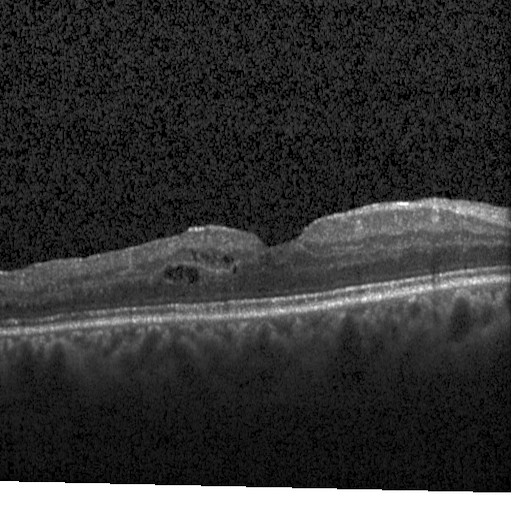
Spectral-domain OCT B-scan: diabetic macular edema (DME).